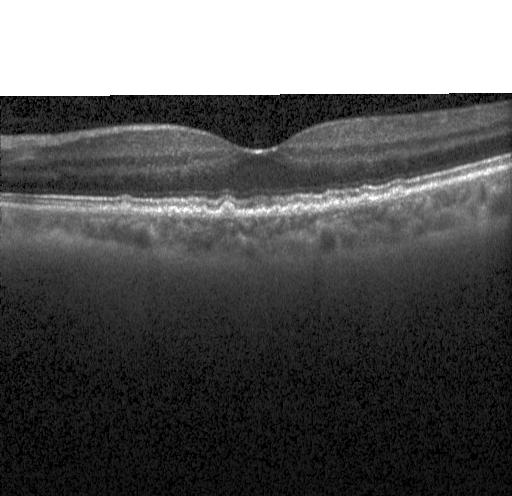
Macular OCT: drusen.